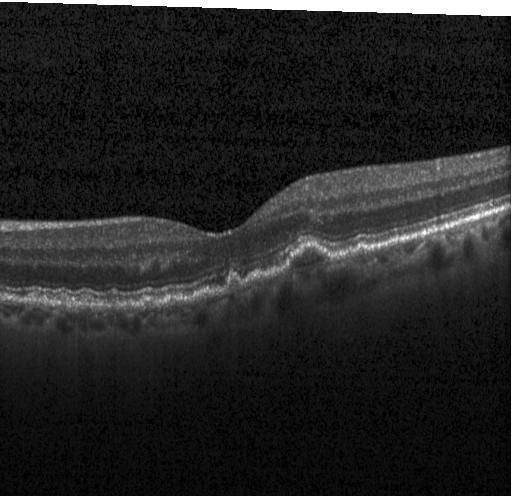
Fovea-centered, optical coherence tomography B-scan — Drusen.